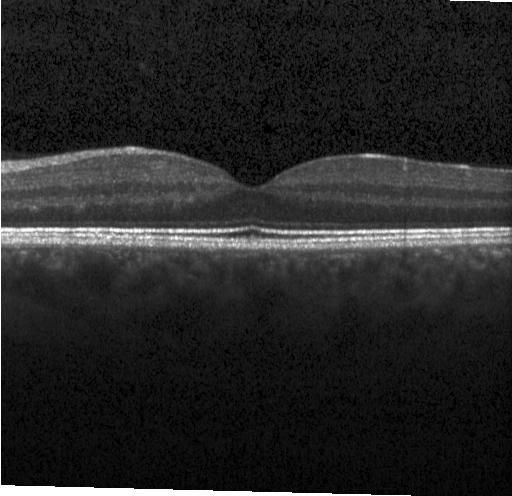 OCT line scan; centered on the fovea; spectral-domain OCT
This B-scan demonstrates no choroidal neovascularization, diabetic macular edema, or drusen.